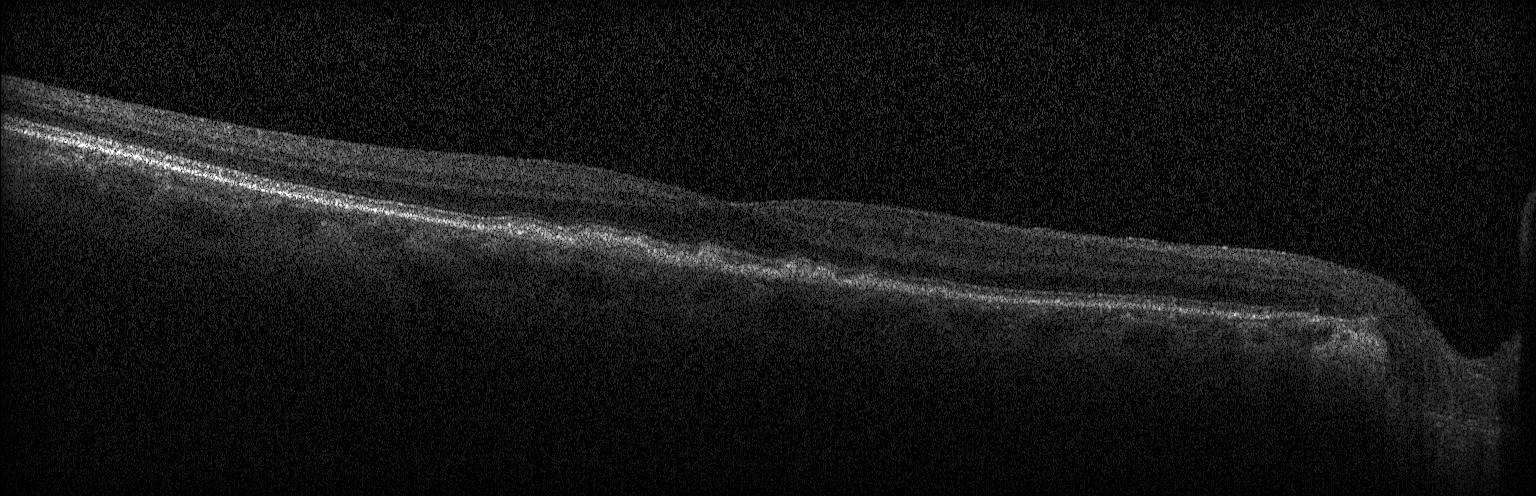
Optical coherence tomography B-scan, spectral-domain optical coherence tomography, instrument: Heidelberg Spectralis
Finding: multiple drusen.